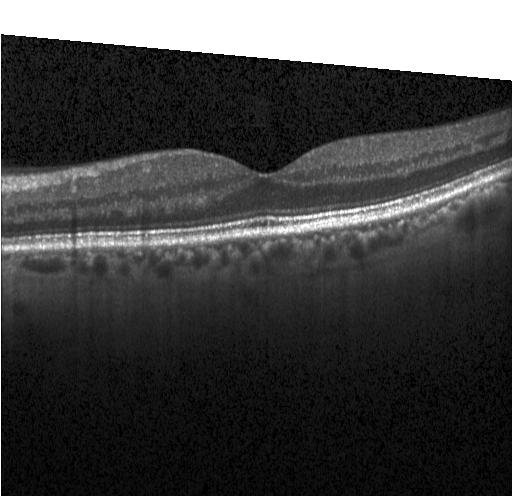
Macular OCT demonstrating neither CNV, DME, nor drusen.